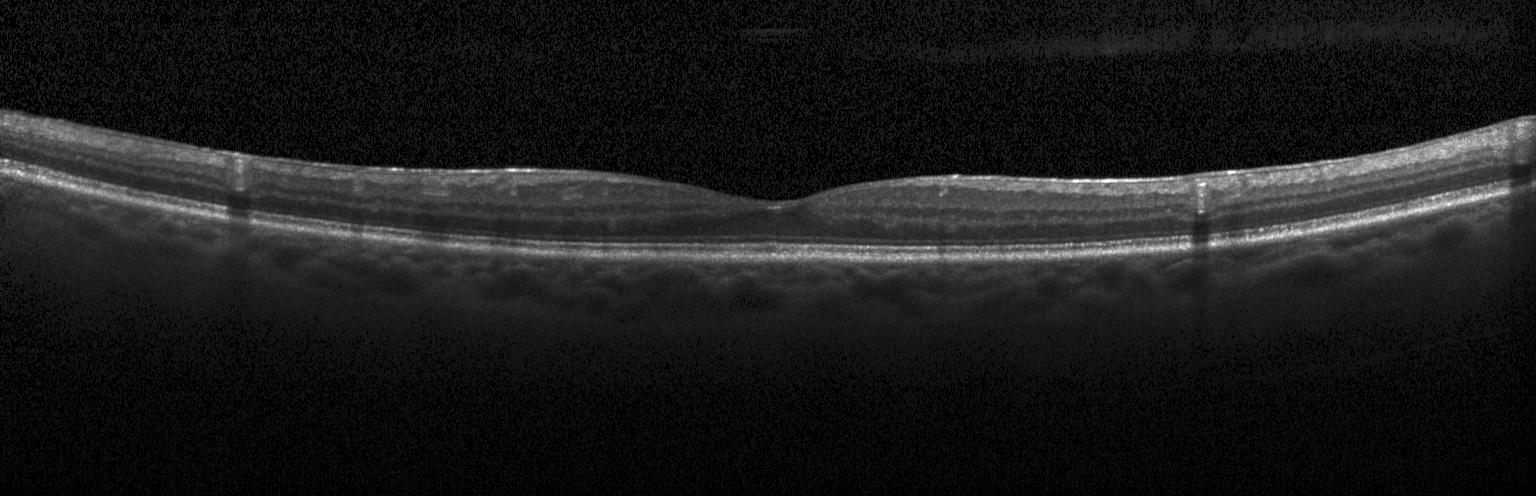
Finding: no evidence of choroidal neovascularization, diabetic macular edema, or drusen.